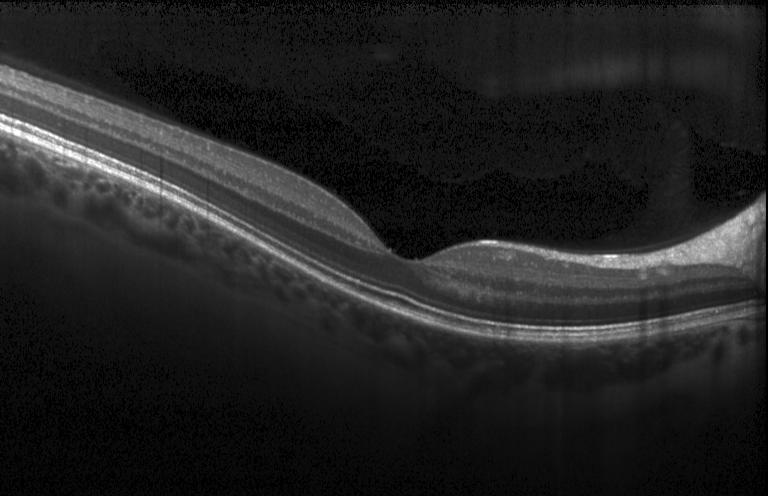 Impression: no CNV, no DME, and no drusen.